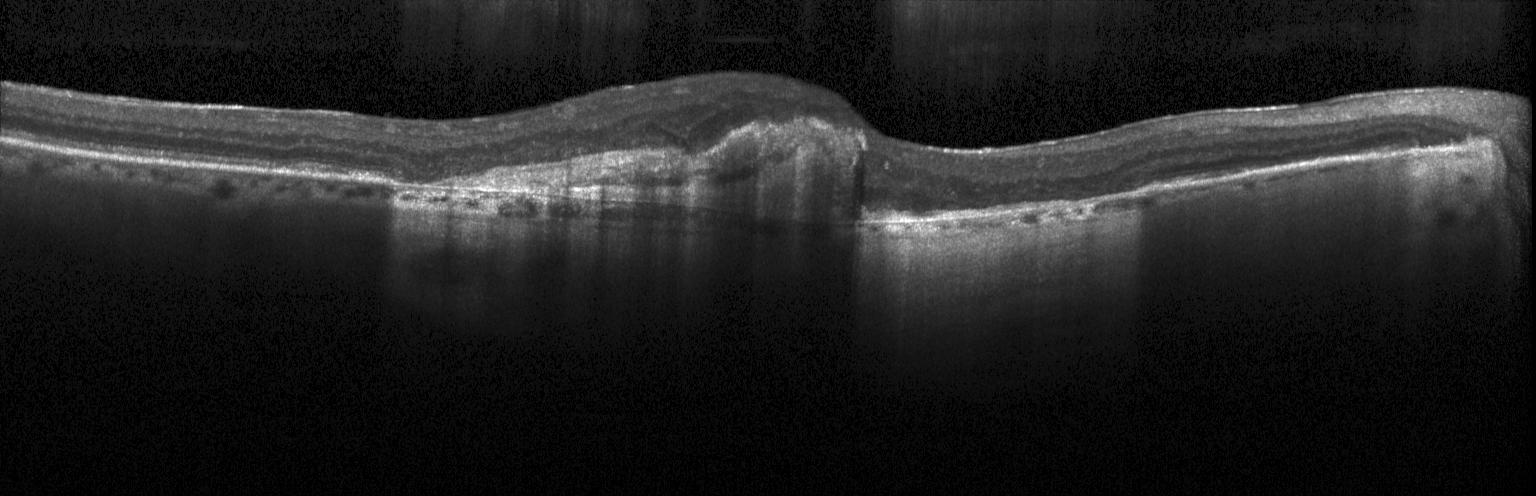

Finding: choroidal neovascularization.